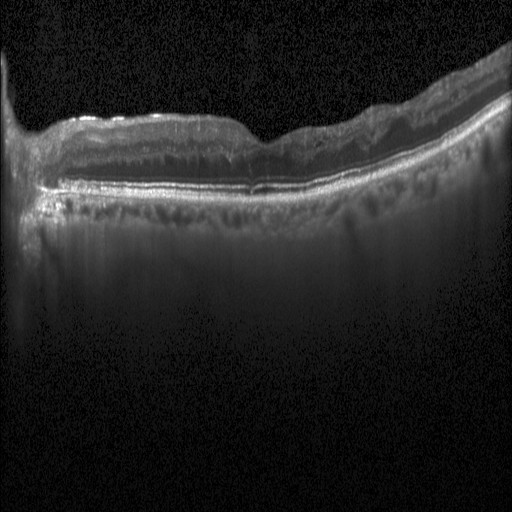 Spectral-domain OCT; acquired on a Heidelberg Spectralis; OCT line scan; centered on the fovea — Finding: diabetic macular edema (DME).